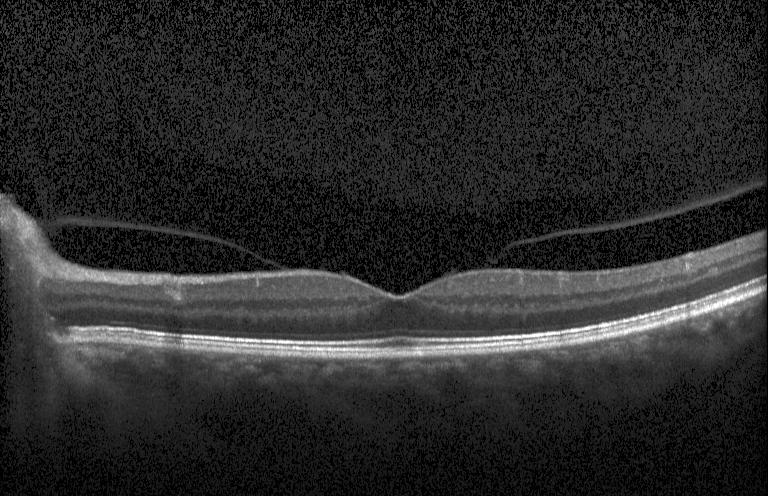

OCT B-scan showing neither CNV, DME, nor drusen.